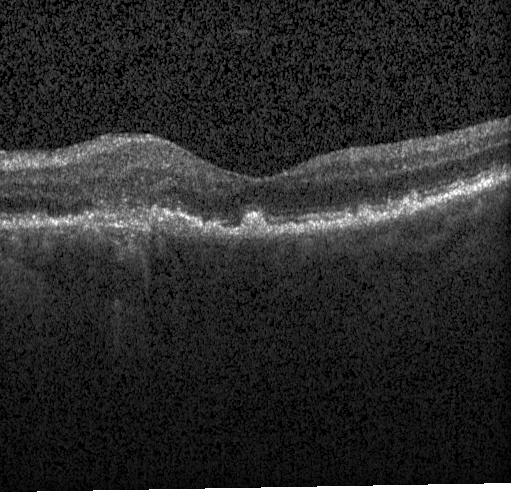 Retinal OCT B-scan. Spectral-domain optical coherence tomography. Macular scan. Impression: a choroidal neovascular membrane.